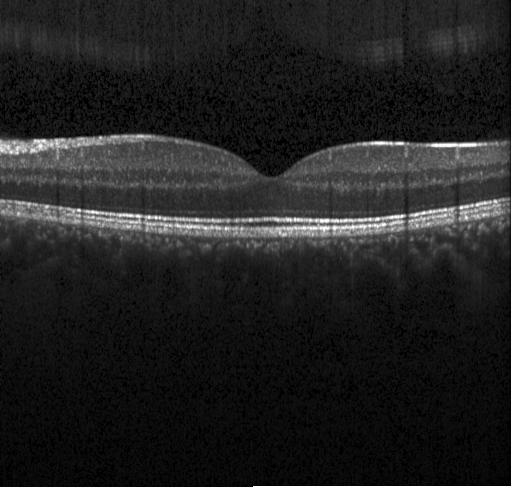 OCT line scan. Horizontal scan through the fovea. SD-OCT.
Impression: neither choroidal neovascularization, diabetic macular edema, nor drusen.